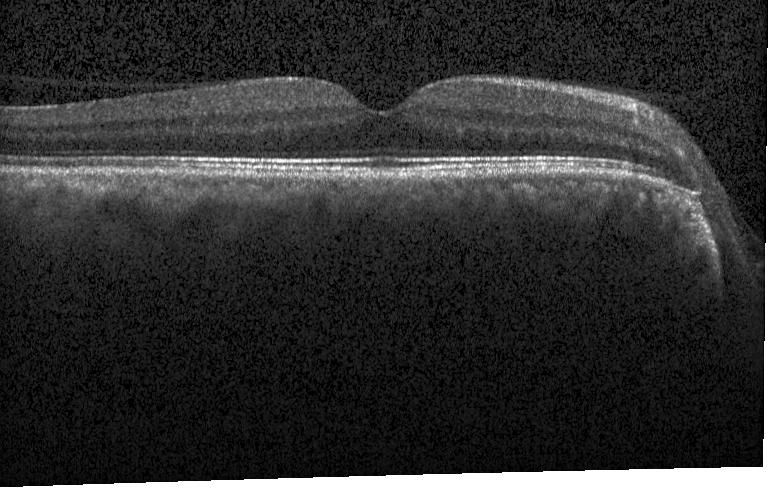
Retinal OCT B-scan, Heidelberg Spectralis, through the macula. Impression: no CNV, DME, or drusen.